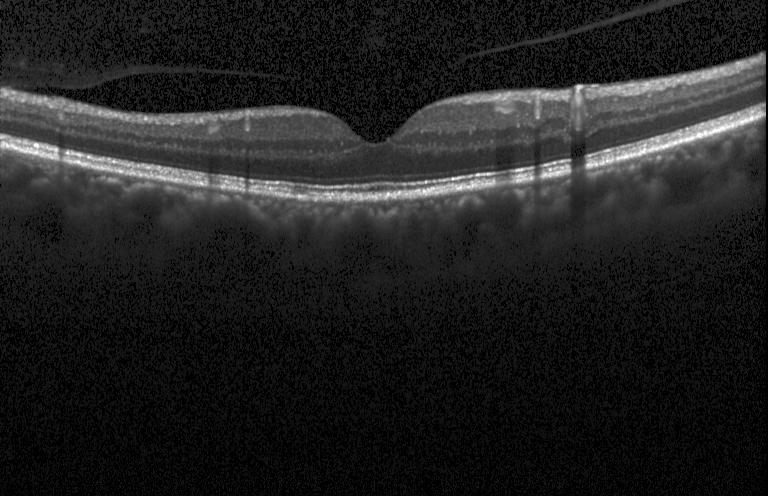 Macular OCT demonstrating no choroidal neovascularization, no diabetic macular edema, and no drusen.